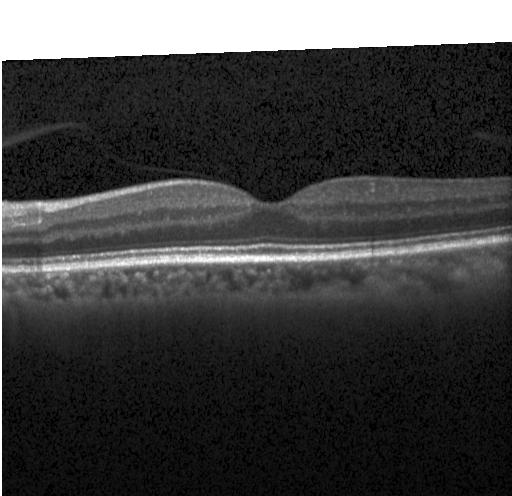 Horizontal scan through the fovea · retinal OCT cross-section
Neither CNV, DME, nor drusen.